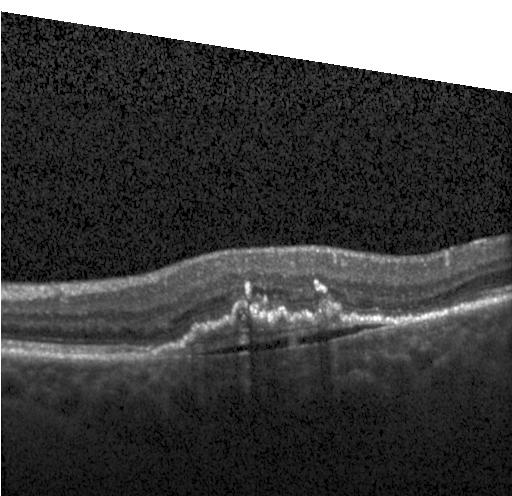 A choroidal neovascular membrane.